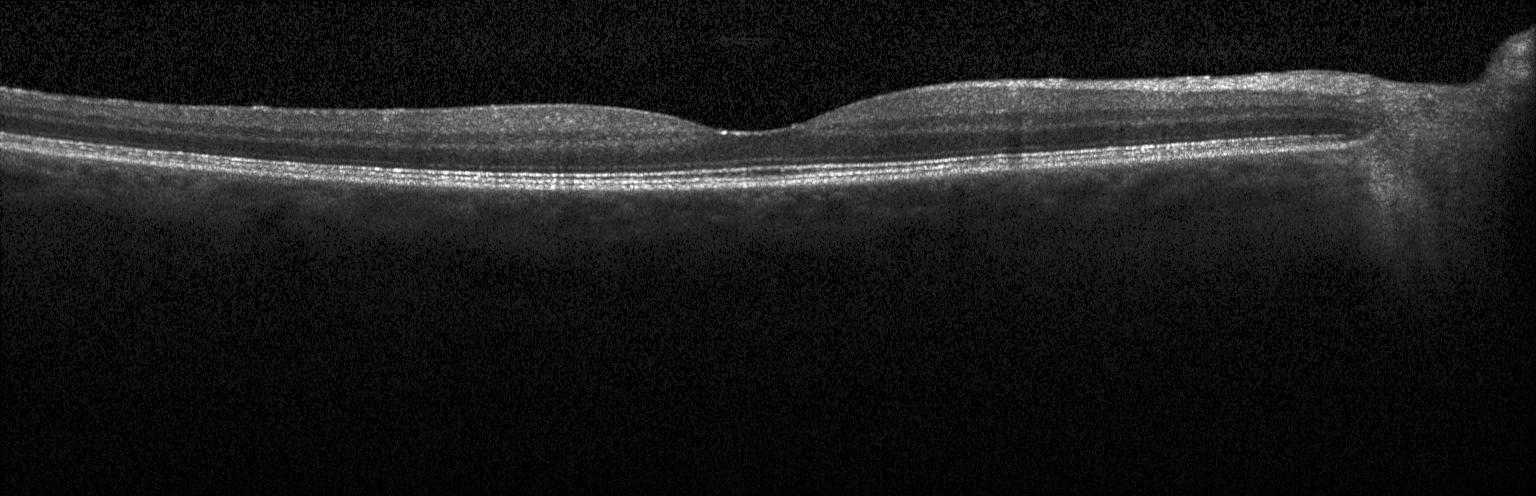 Dx: neither choroidal neovascularization, diabetic macular edema, nor drusen.